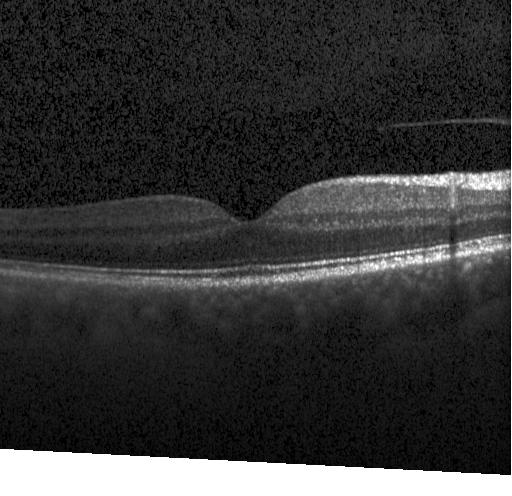
Macular OCT: no evidence of choroidal neovascularization, diabetic macular edema, or drusen.